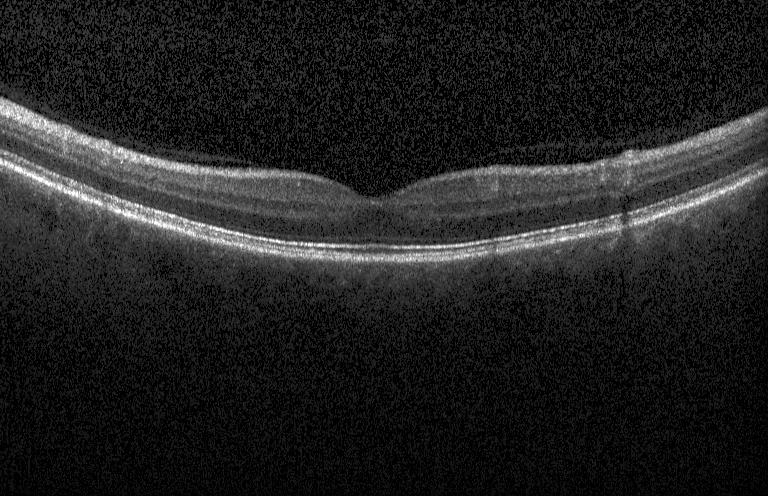

Acquired on a Heidelberg Spectralis. Spectral-domain optical coherence tomography. Horizontal scan through the fovea. Retinal OCT cross-section
Neither choroidal neovascularization, diabetic macular edema, nor drusen.